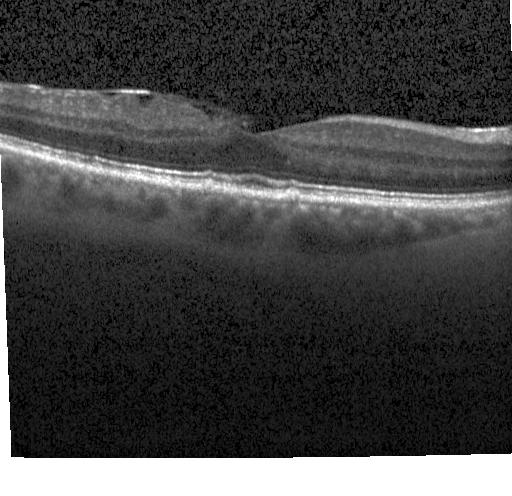
Macular OCT demonstrating sub-RPE drusenoid deposits.